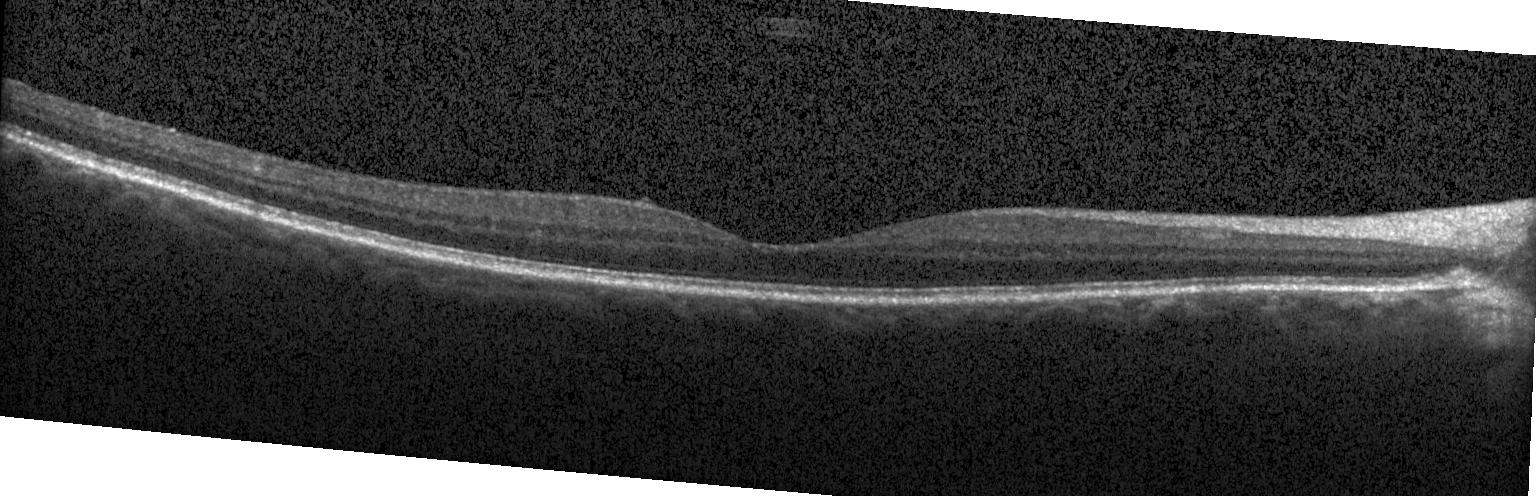
Finding: no choroidal neovascularization, diabetic macular edema, or drusen.